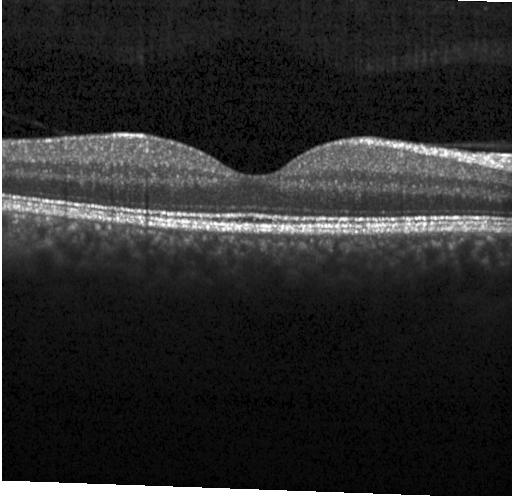

Heidelberg Spectralis OCT system; retinal OCT cross-section; macular scan; SD-OCT — Diagnosis: neither choroidal neovascularization, diabetic macular edema, nor drusen.